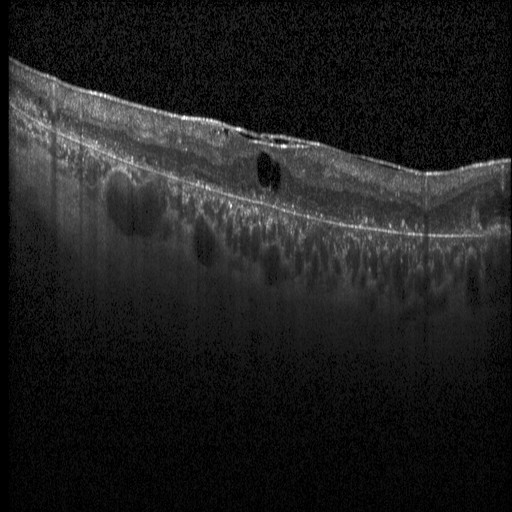 OCT B-scan, acquired on a Heidelberg Spectralis, macular scan
Diagnosis: diabetic macular edema.